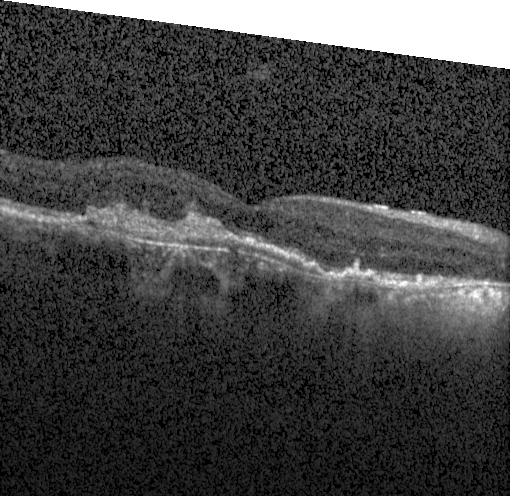

Diagnosis: a choroidal neovascular membrane.